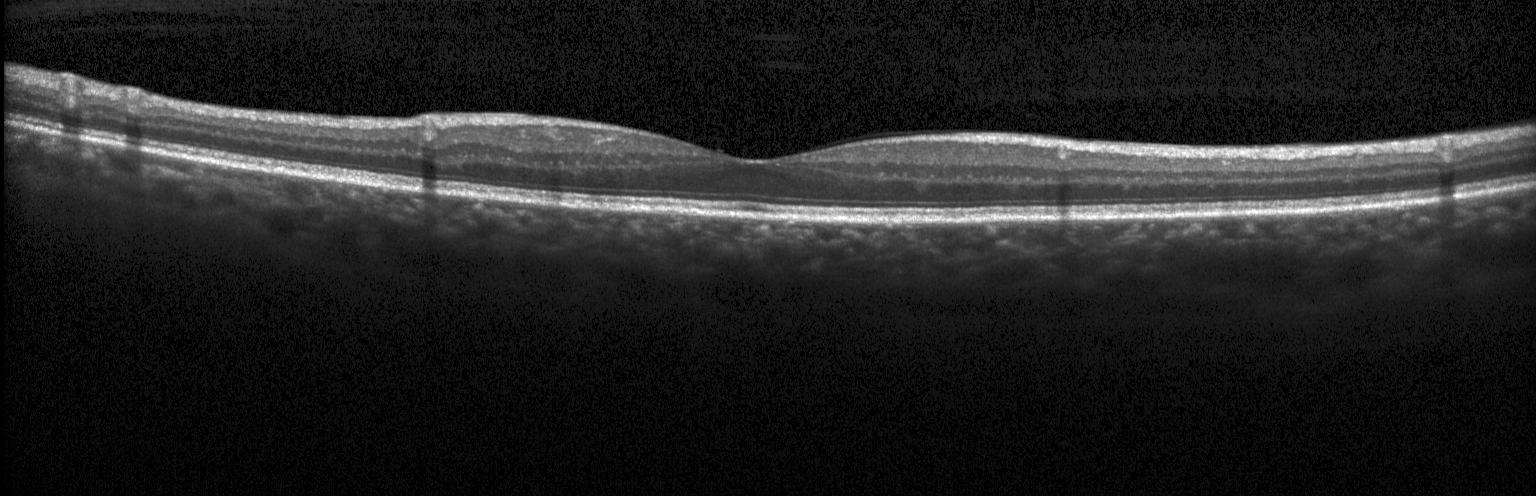

OCT line scan. No CNV, DME, or drusen.